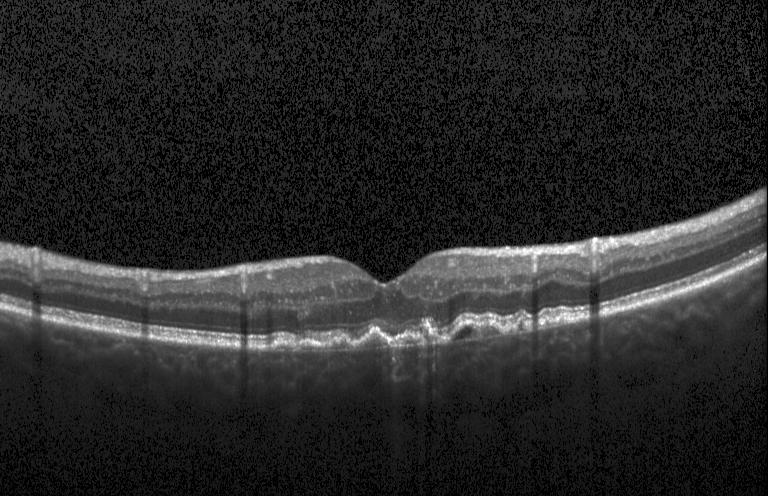 Retinal OCT cross-section
Dx: drusen.